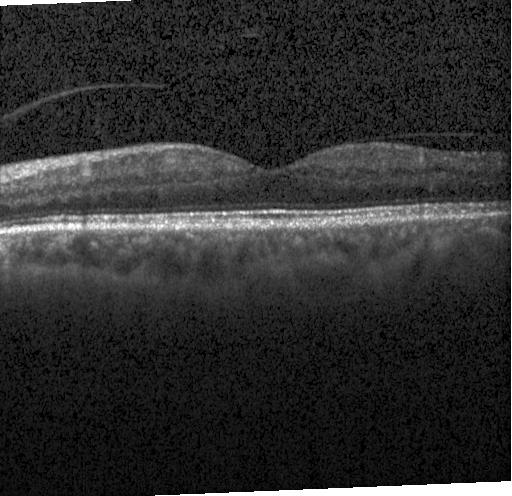
OCT line scan
This B-scan demonstrates no CNV, DME, or drusen.